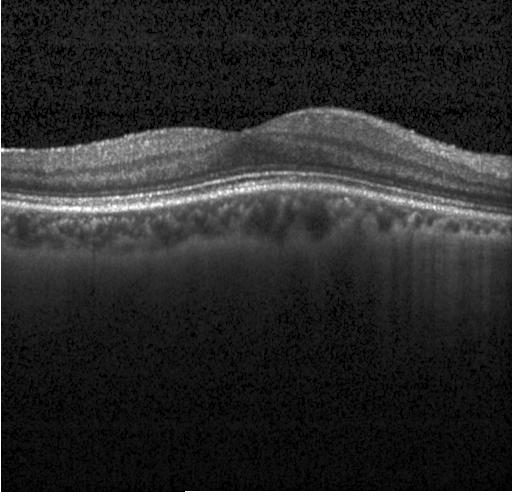

Retinal OCT B-scan; acquired on a Heidelberg Spectralis — OCT finding: no evidence of choroidal neovascularization, diabetic macular edema, or drusen.